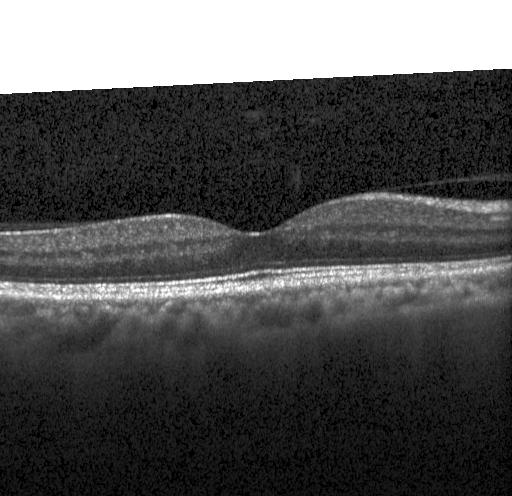 The scan shows no CNV, DME, or drusen.